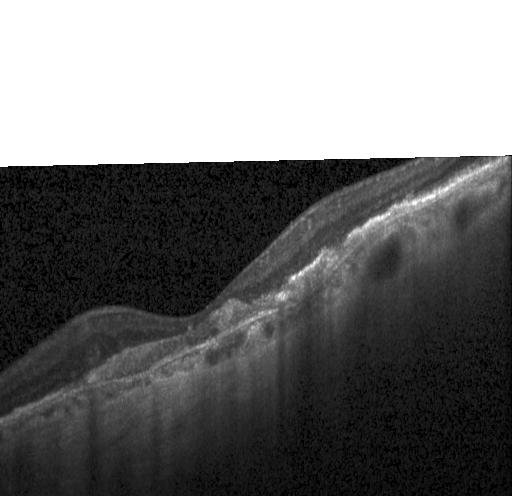
The scan shows CNV.